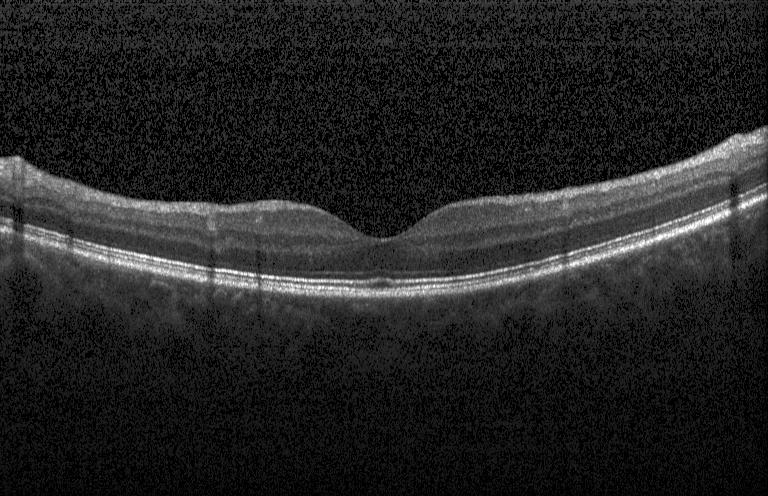

Diagnosis: no choroidal neovascularization, no diabetic macular edema, and no drusen.